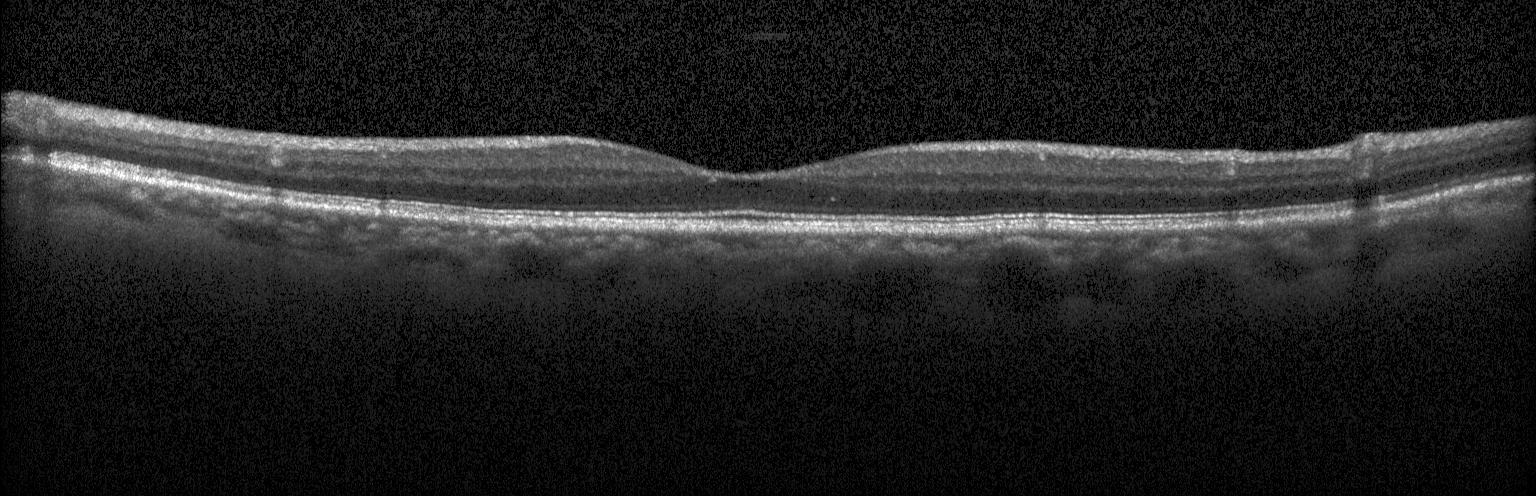
Retinal OCT cross-section.
OCT finding: no evidence of choroidal neovascularization, diabetic macular edema, or drusen.